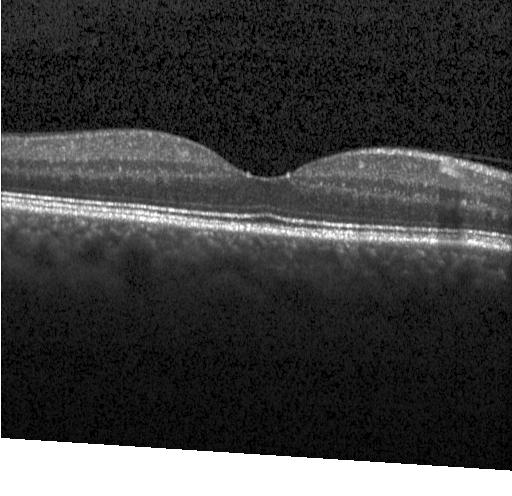 Impression: no choroidal neovascularization, no diabetic macular edema, and no drusen.